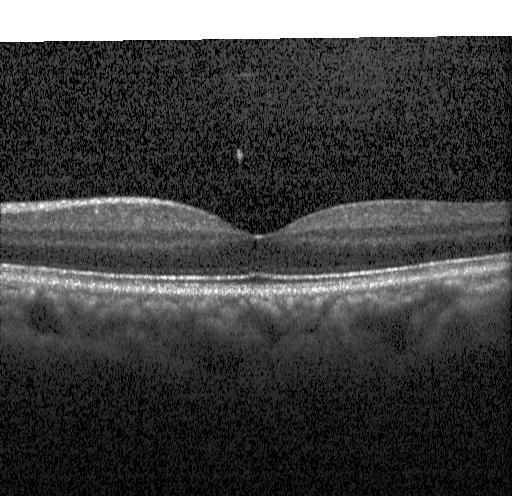
Spectral-domain optical coherence tomography · optical coherence tomography scan · macular scan. The scan shows no evidence of CNV, DME, or drusen.